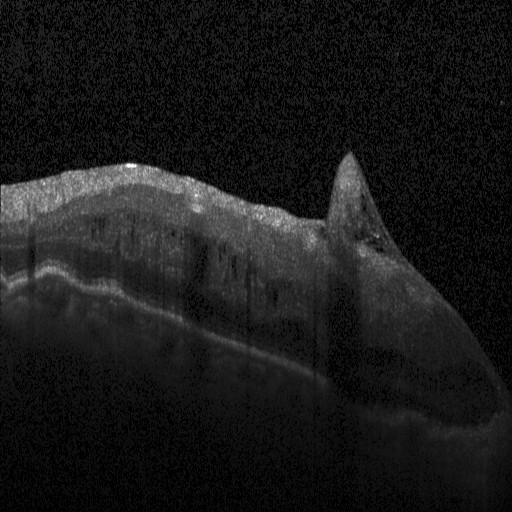

Diagnosis: diabetic macular edema (DME).